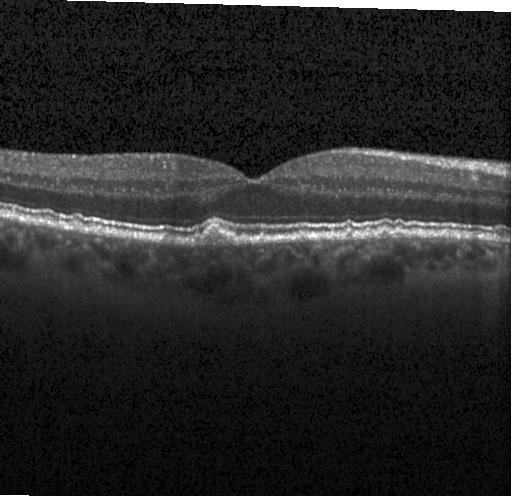

The scan shows multiple drusen.